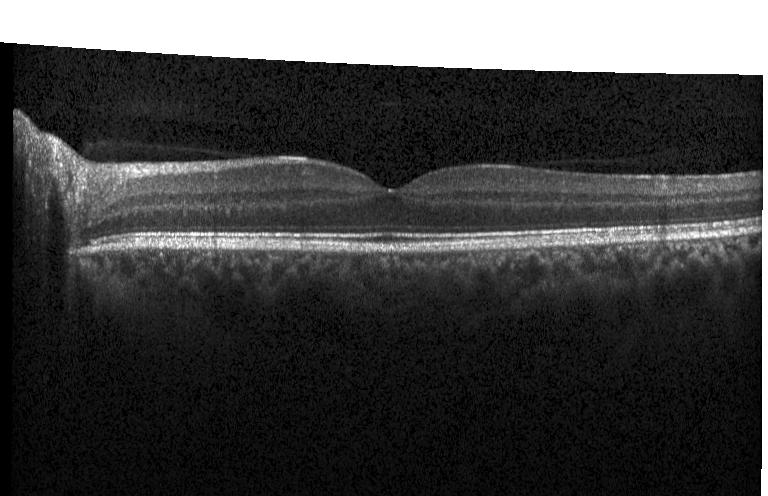 Finding: neither choroidal neovascularization, diabetic macular edema, nor drusen.